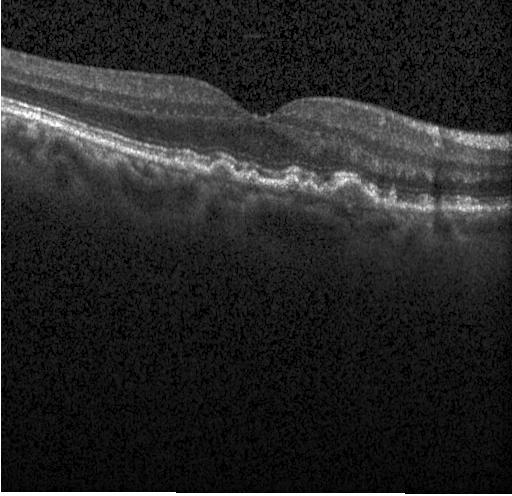
Acquired on a Heidelberg Spectralis, fovea-centered, optical coherence tomography B-scan, spectral-domain OCT. Finding: multiple drusen.